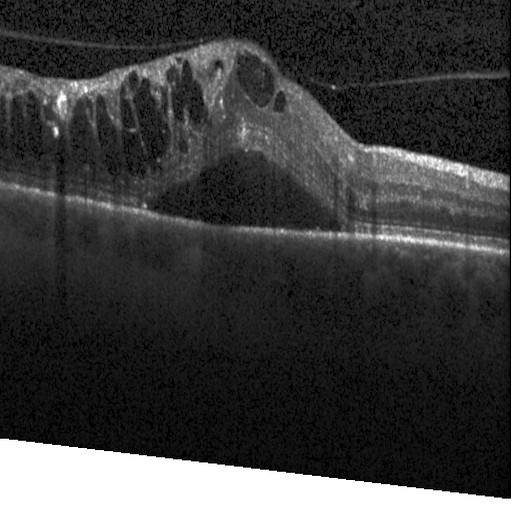

Retinal OCT cross-section · macular scan · spectral-domain OCT.
This B-scan demonstrates diabetic macular edema (DME).